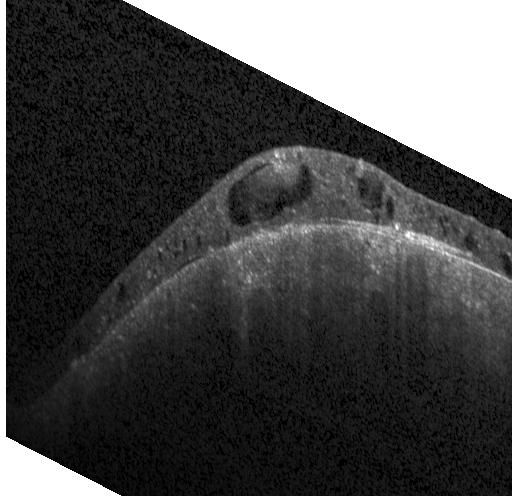
Retinal OCT B-scan; SD-OCT; instrument: Heidelberg Spectralis
Dx: diabetic macular edema (DME).